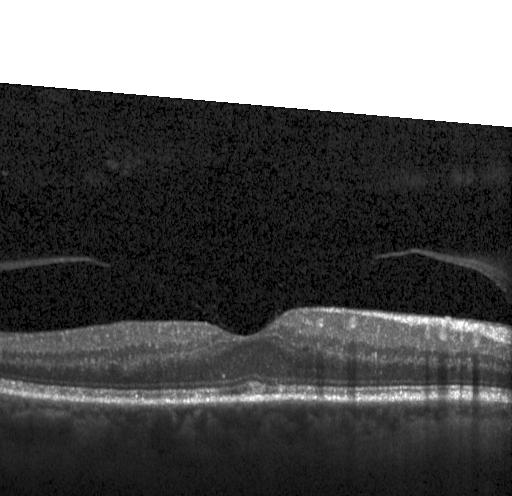

Retinal OCT B-scan, SD-OCT.
Macular OCT: no evidence of choroidal neovascularization, diabetic macular edema, or drusen.